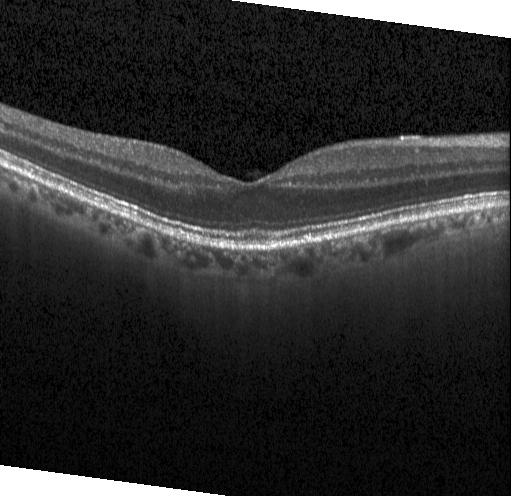 The scan shows no evidence of choroidal neovascularization, diabetic macular edema, or drusen.